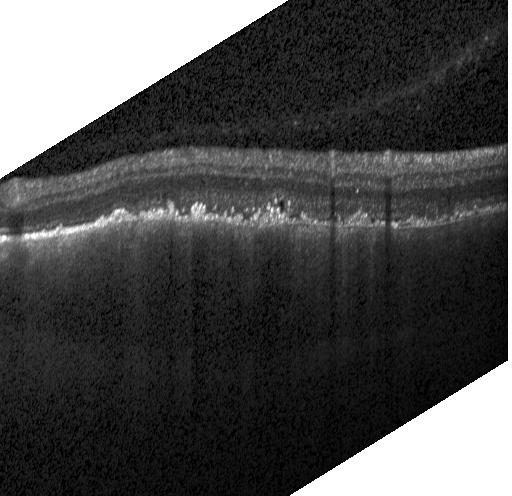 OCT scan showing CNV.